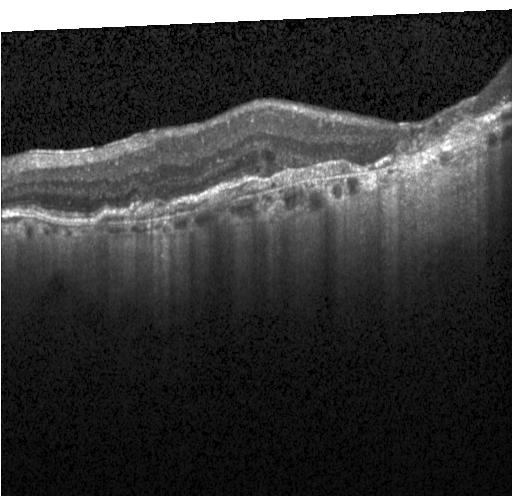

Optical coherence tomography scan. Heidelberg Spectralis — Choroidal neovascularization.